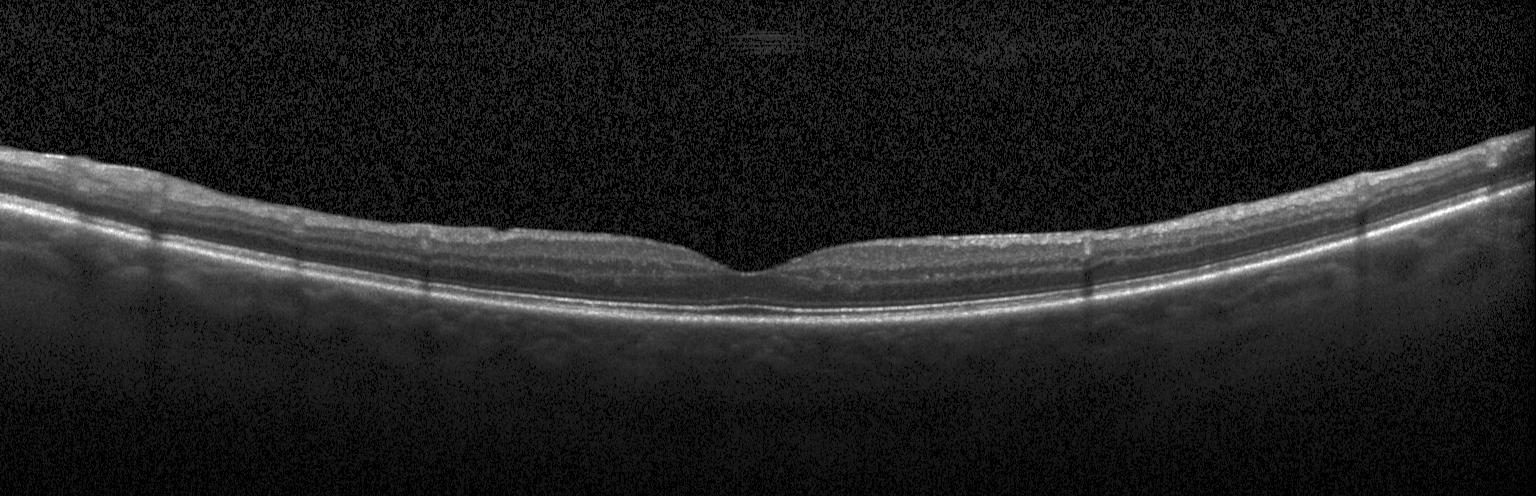 Through the macula · instrument: Heidelberg Spectralis · SD-OCT · retinal OCT B-scan — Impression: no evidence of CNV, DME, or drusen.